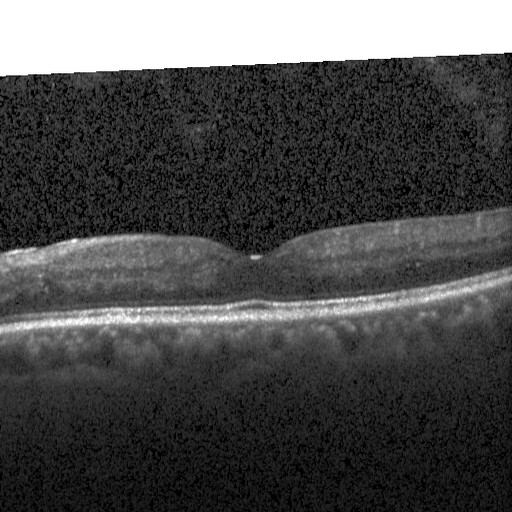 Finding: diabetic macular edema (DME).